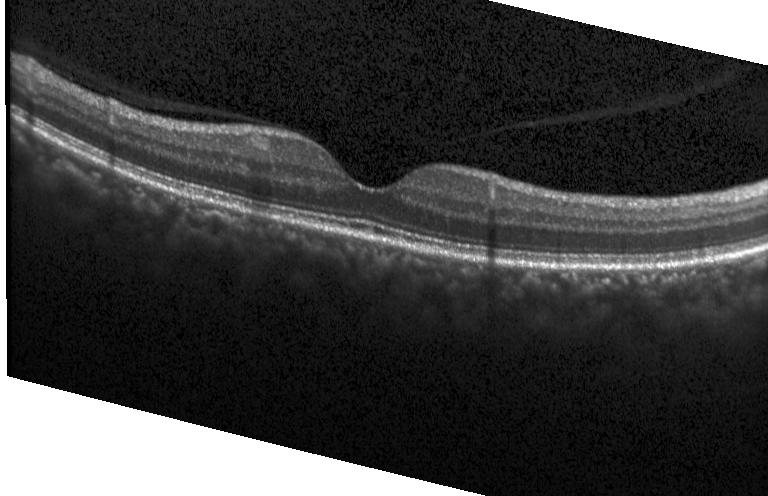
Diagnosis: no choroidal neovascularization, no diabetic macular edema, and no drusen.